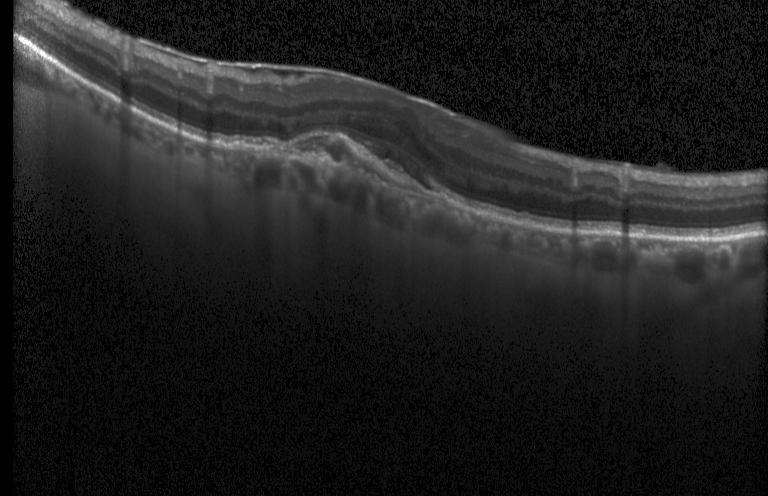 Finding: a choroidal neovascular membrane.